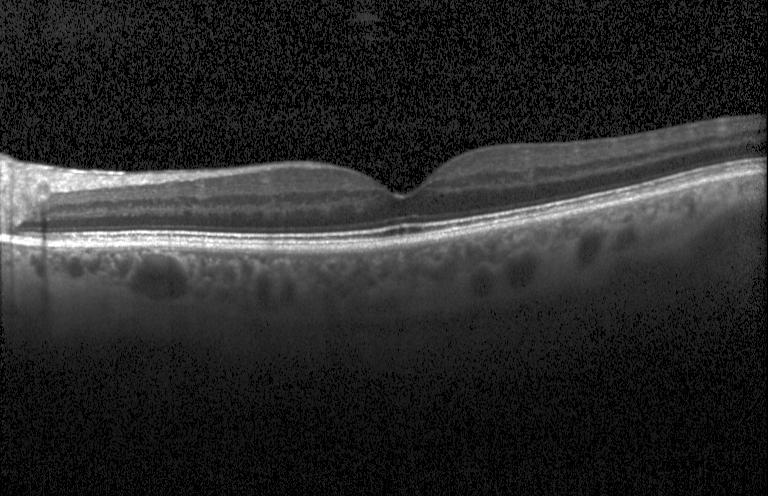 Instrument: Heidelberg Spectralis · centered on the fovea · retinal OCT B-scan · spectral-domain optical coherence tomography. This B-scan demonstrates no choroidal neovascularization, diabetic macular edema, or drusen.